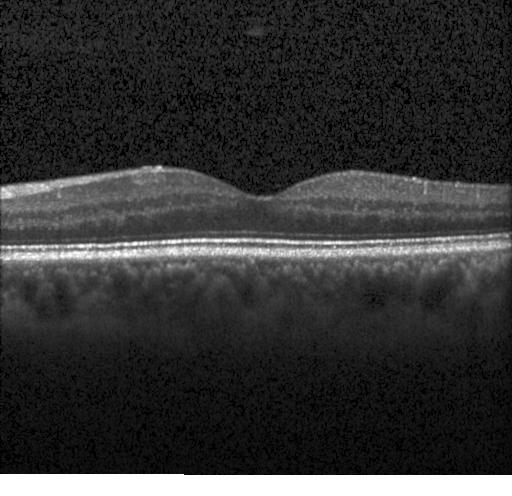 Optical coherence tomography scan.
Assessment: no evidence of choroidal neovascularization, diabetic macular edema, or drusen.